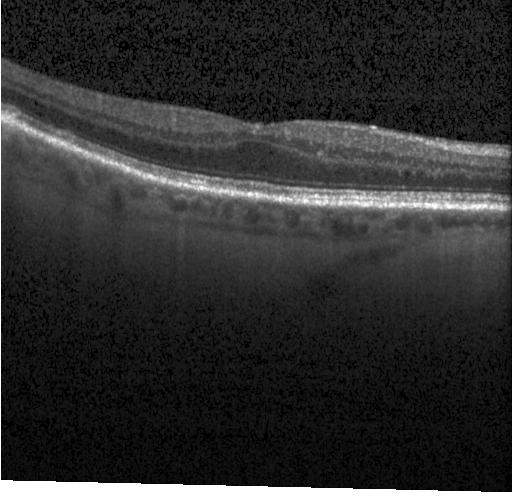
OCT B-scan
Assessment: no choroidal neovascularization, no diabetic macular edema, and no drusen.